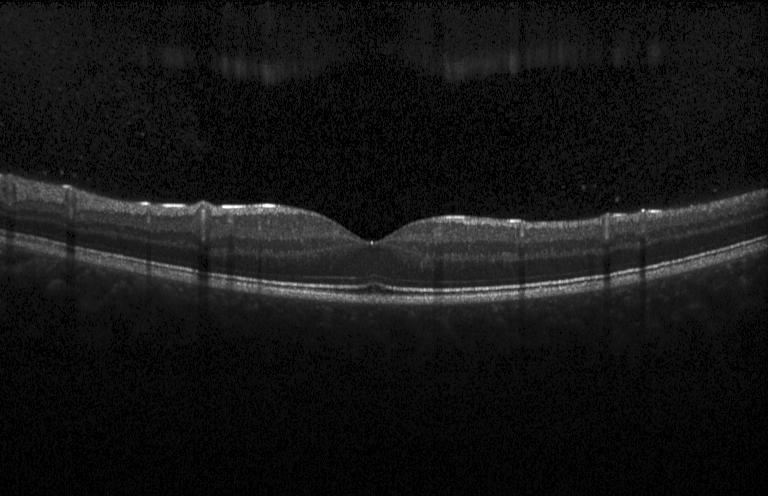 Instrument: Heidelberg Spectralis, optical coherence tomography B-scan, fovea-centered
This B-scan demonstrates no choroidal neovascularization, diabetic macular edema, or drusen.